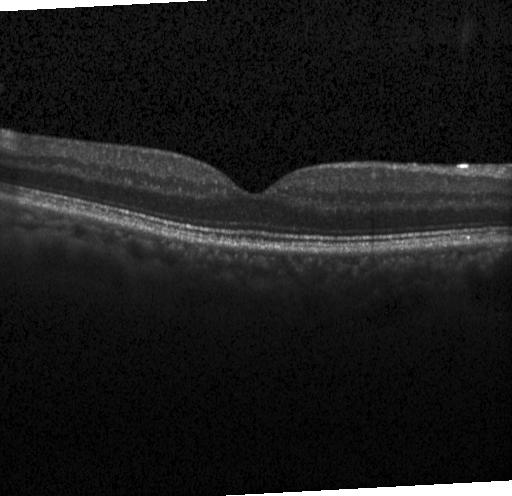
Macular OCT: no choroidal neovascularization, no diabetic macular edema, and no drusen.